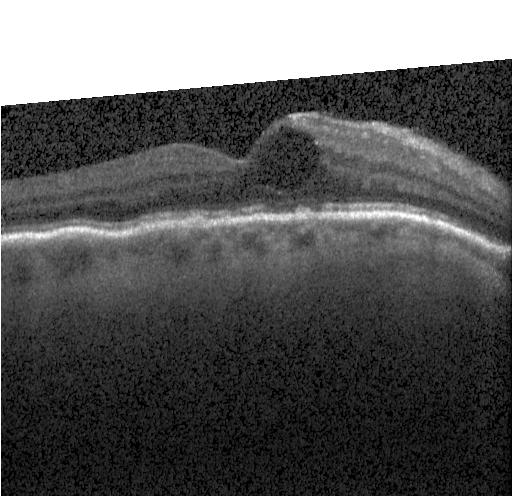
OCT finding: DME.